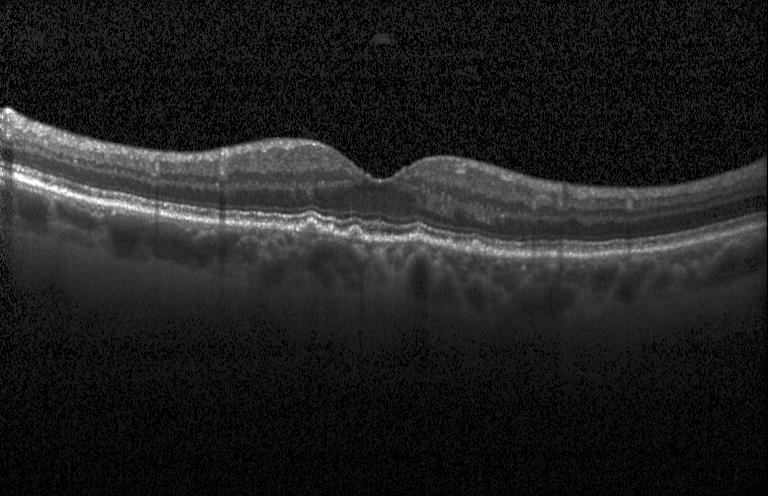

Diagnosis: multiple drusen.